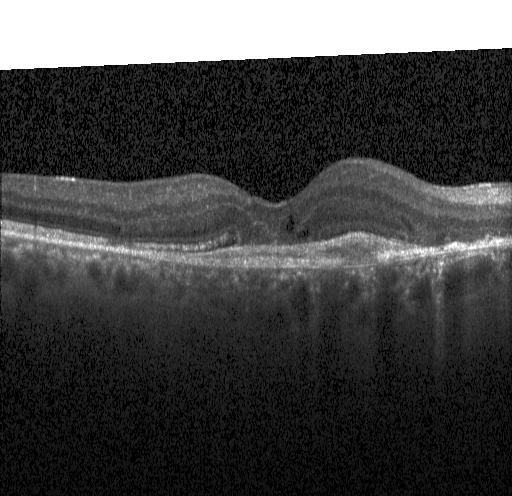 Acquired on a Heidelberg Spectralis, SD-OCT, retinal OCT cross-section. Diagnosis: a choroidal neovascular membrane.